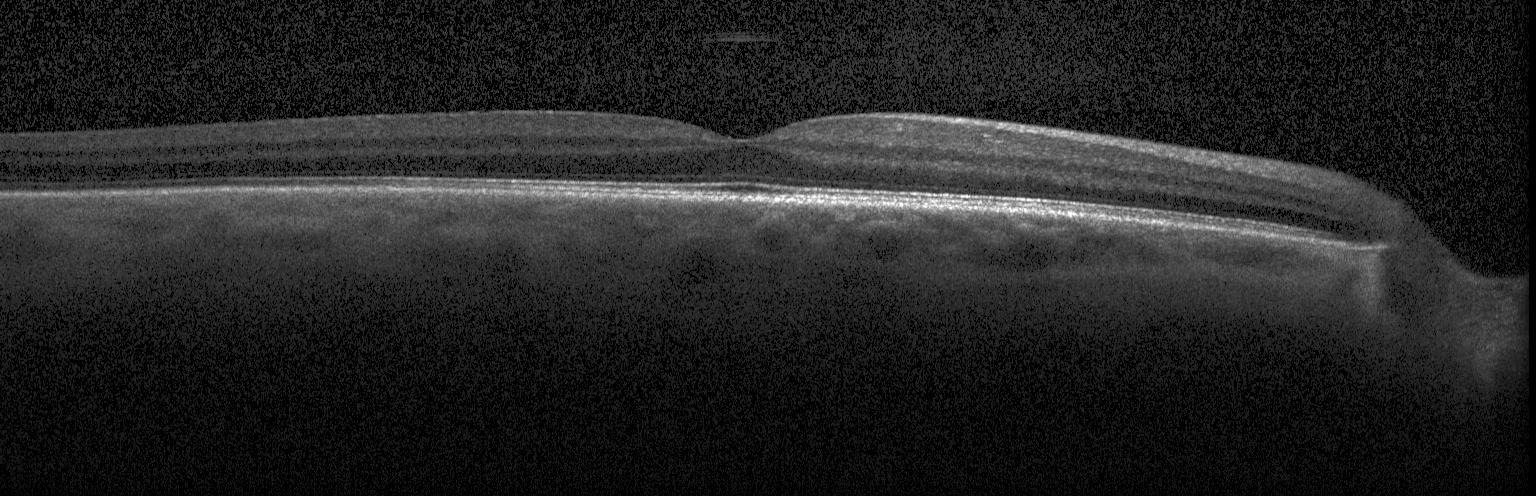
Instrument: Heidelberg Spectralis; through the macula; OCT line scan; spectral-domain OCT — The scan shows no evidence of CNV, DME, or drusen.